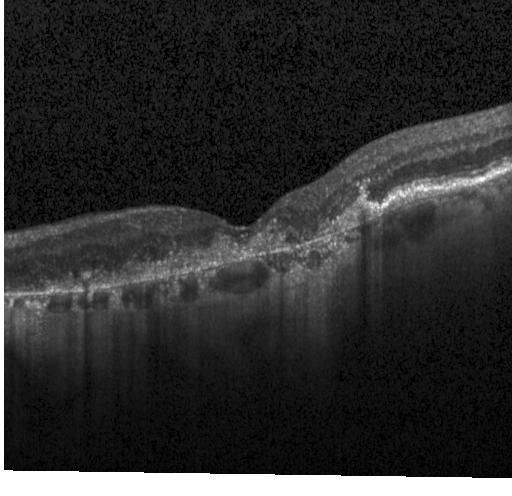
Spectral-domain optical coherence tomography. Through the macula. Heidelberg Spectralis. Optical coherence tomography scan
Diagnosis: a choroidal neovascular membrane.